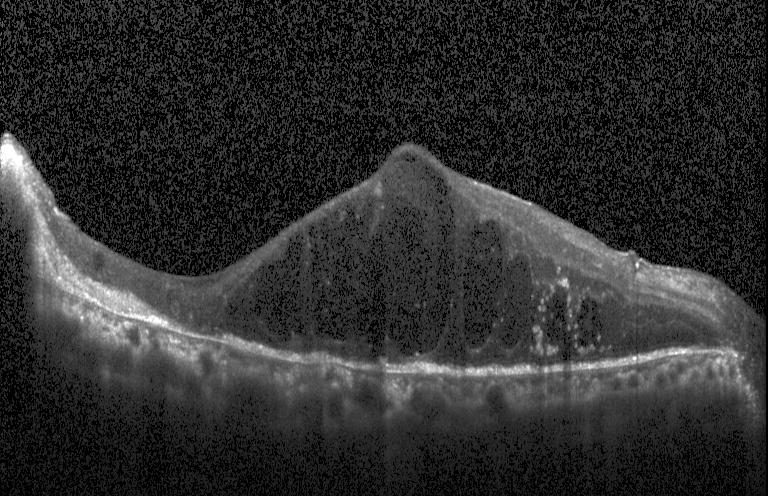
Finding: diabetic macular edema (DME).